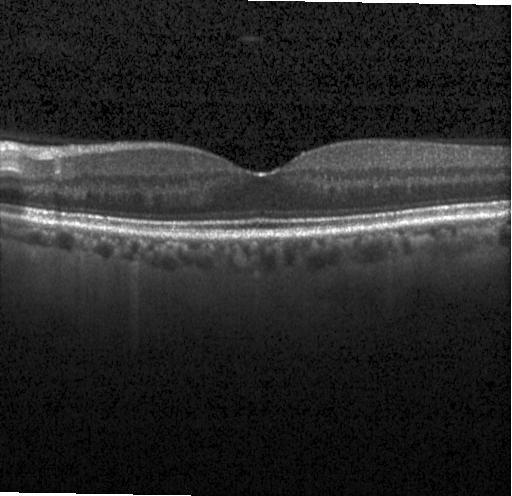 Macular OCT: neither CNV, DME, nor drusen.